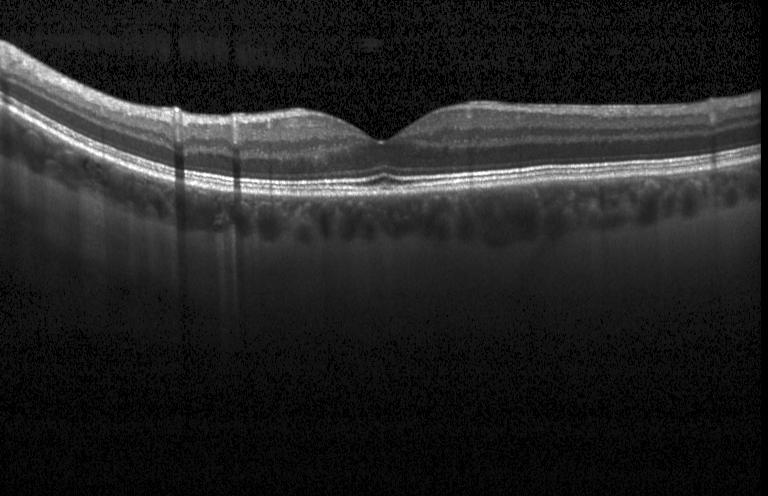

Dx: no evidence of CNV, DME, or drusen.